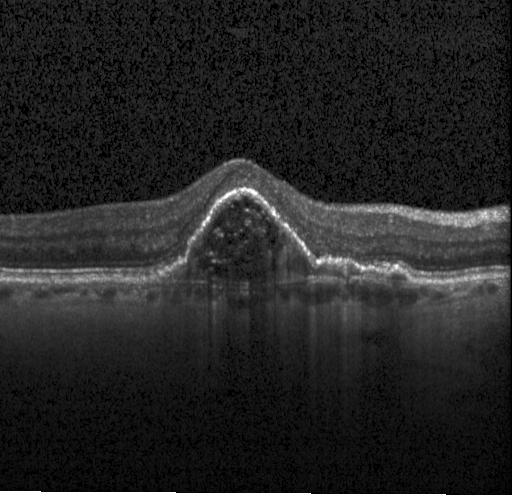
Spectral-domain OCT. Through the macula. Heidelberg Spectralis OCT system. OCT B-scan
This B-scan demonstrates CNV.